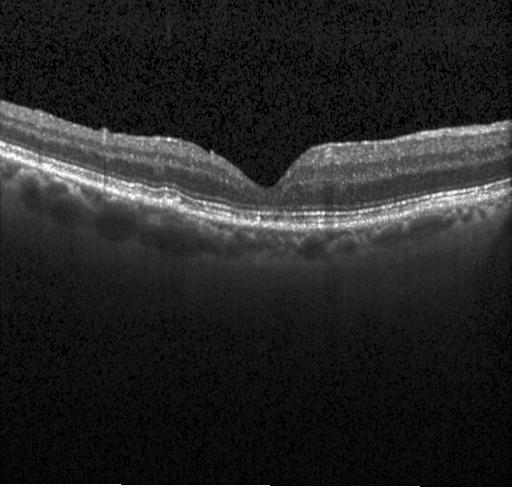
Retinal OCT cross-section. Heidelberg Spectralis OCT system. Fovea-centered — The scan shows multiple drusen.